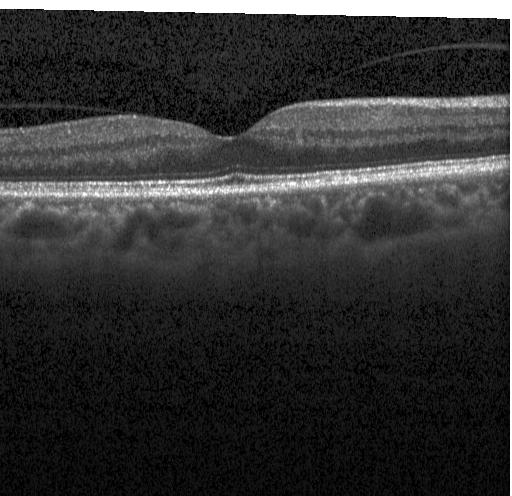 OCT B-scan · Heidelberg Spectralis OCT system · macular scan · spectral-domain optical coherence tomography. Assessment: no evidence of choroidal neovascularization, diabetic macular edema, or drusen.